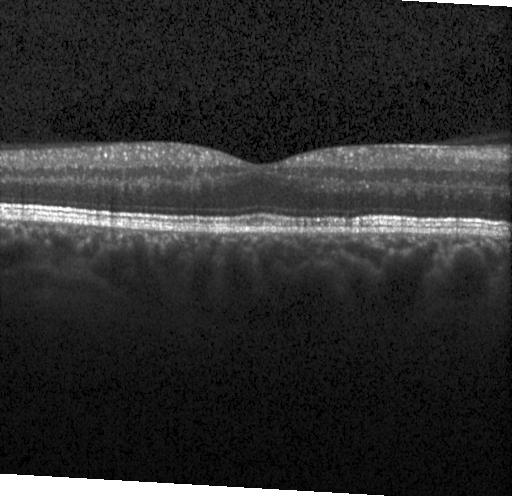
OCT scan showing no choroidal neovascularization, diabetic macular edema, or drusen.